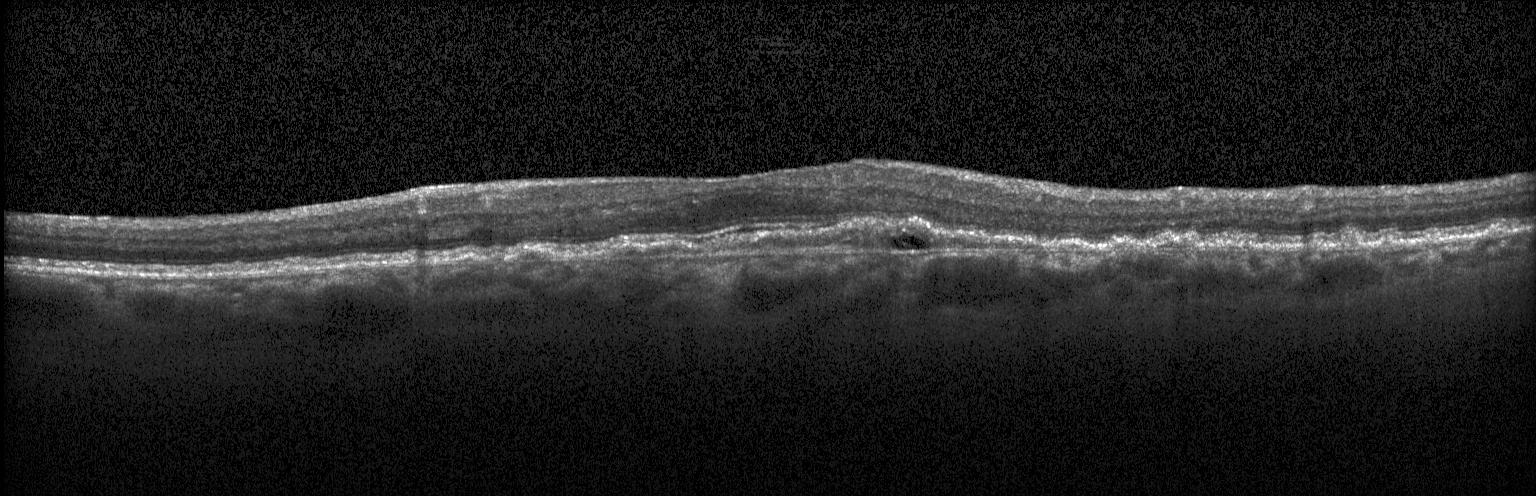
The scan shows a choroidal neovascular membrane.